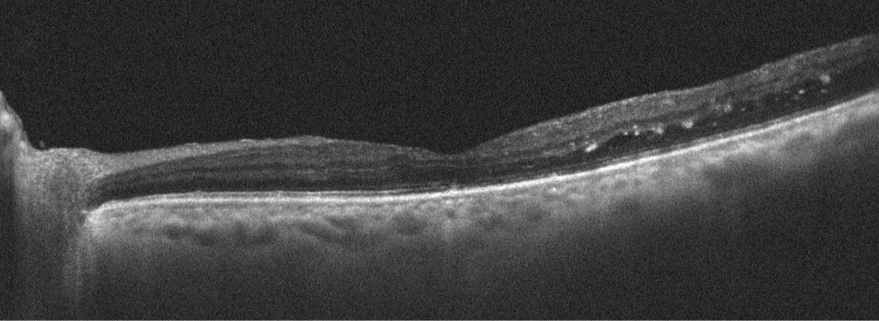 OCT finding: diabetic macular edema (DME).